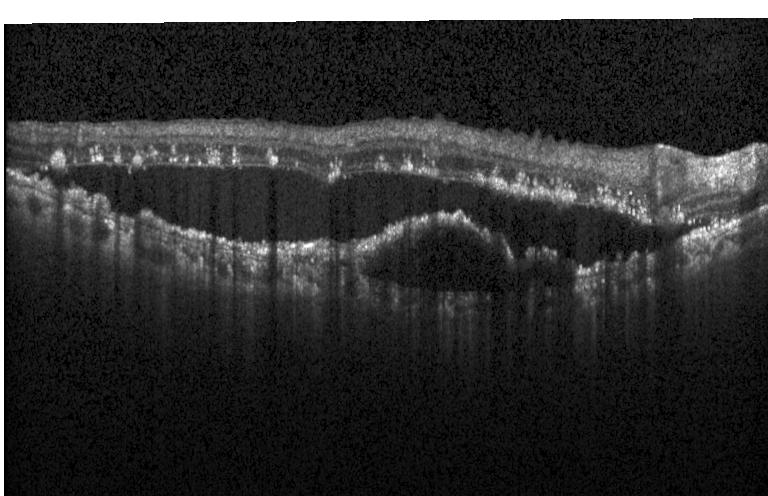 Assessment: a choroidal neovascular membrane.